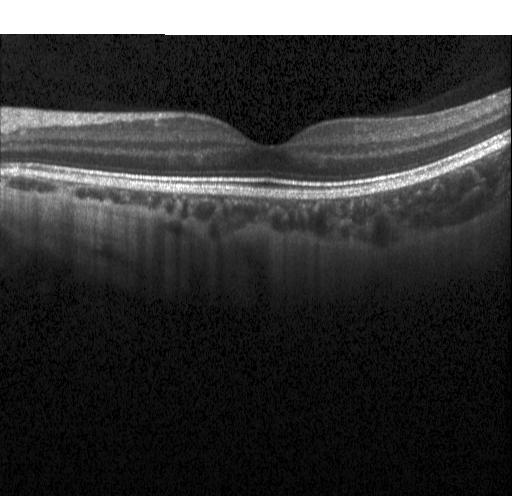

Spectral-domain OCT. Optical coherence tomography B-scan. Heidelberg Spectralis OCT system — Diagnosis: neither choroidal neovascularization, diabetic macular edema, nor drusen.